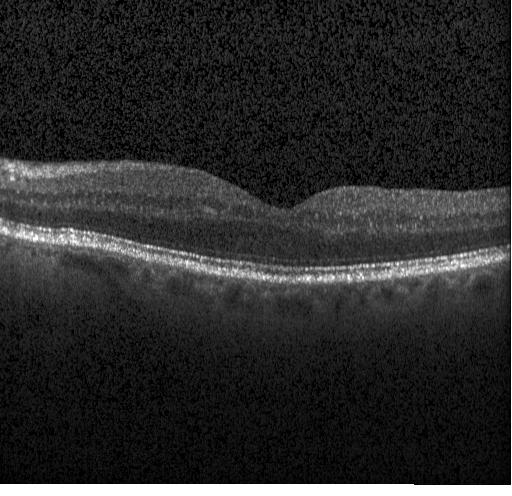

Acquired on a Heidelberg Spectralis. Retinal OCT cross-section — Assessment: no choroidal neovascularization, no diabetic macular edema, and no drusen.